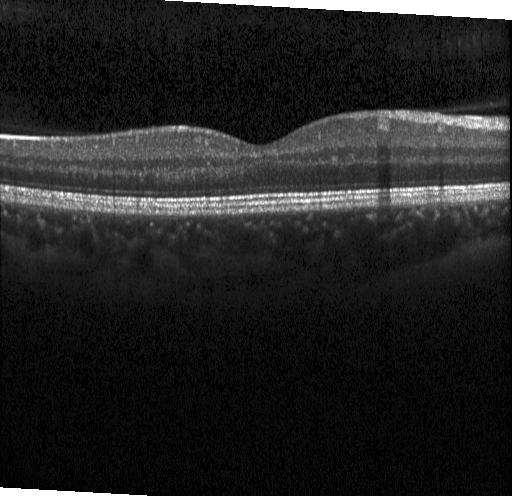 Retinal OCT B-scan.
Finding: no evidence of choroidal neovascularization, diabetic macular edema, or drusen.